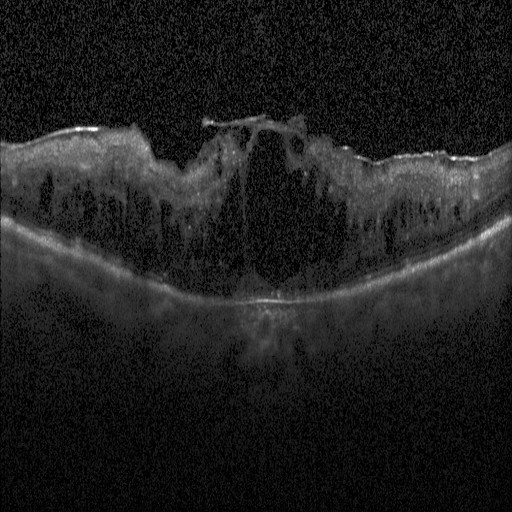
OCT B-scan. Acquired on a Heidelberg Spectralis. This B-scan demonstrates DME.